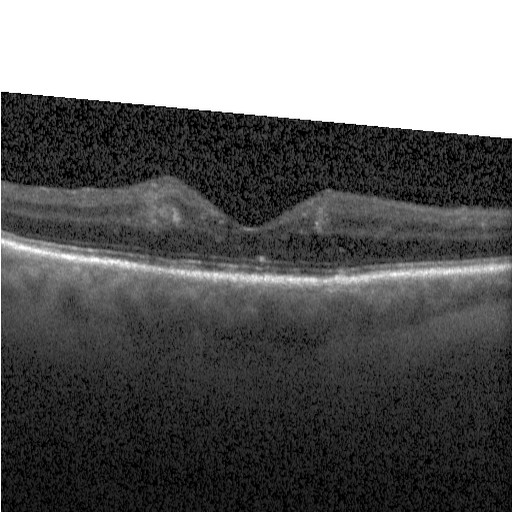

Macular scan, instrument: Heidelberg Spectralis, optical coherence tomography scan. Finding: diabetic macular edema (DME).